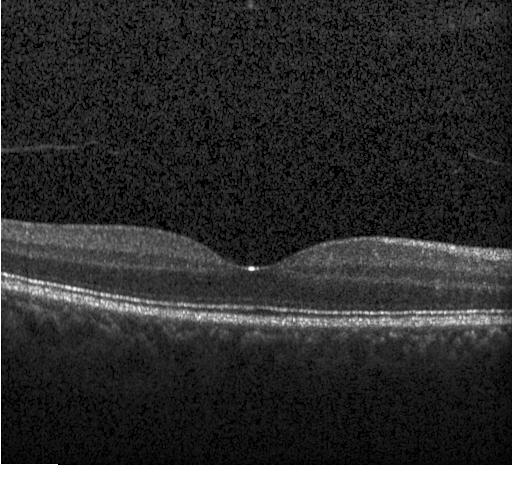 Macular OCT: no evidence of choroidal neovascularization, diabetic macular edema, or drusen.